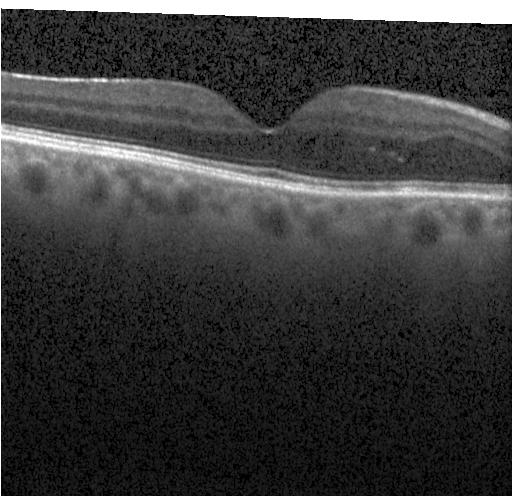 Acquired on a Heidelberg Spectralis · spectral-domain optical coherence tomography · retinal OCT B-scan
Finding: diabetic macular edema (DME).